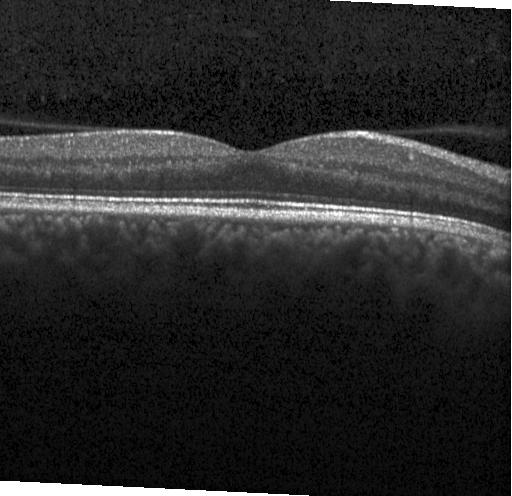 Retinal OCT B-scan, SD-OCT, fovea-centered, instrument: Heidelberg Spectralis.
Neither choroidal neovascularization, diabetic macular edema, nor drusen.